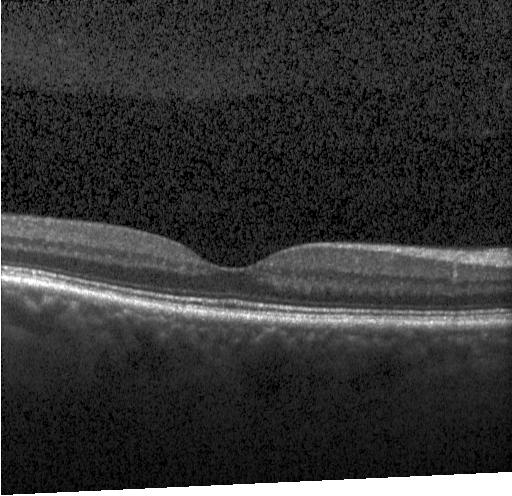
Dx: no CNV, no DME, and no drusen.